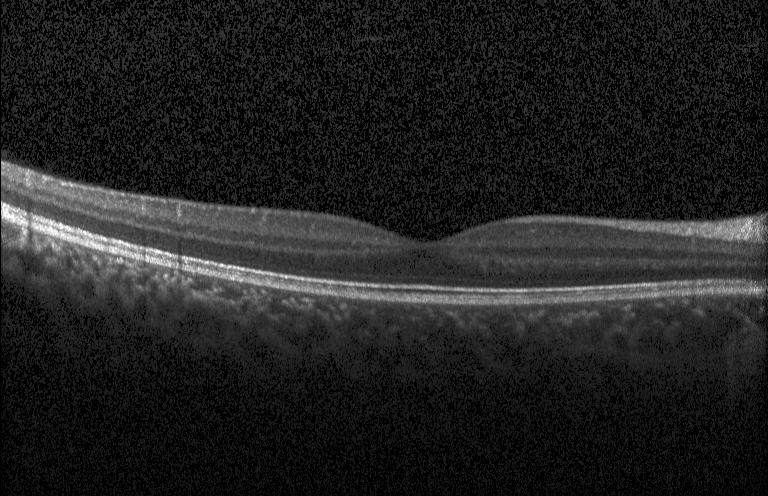 OCT finding: neither choroidal neovascularization, diabetic macular edema, nor drusen.